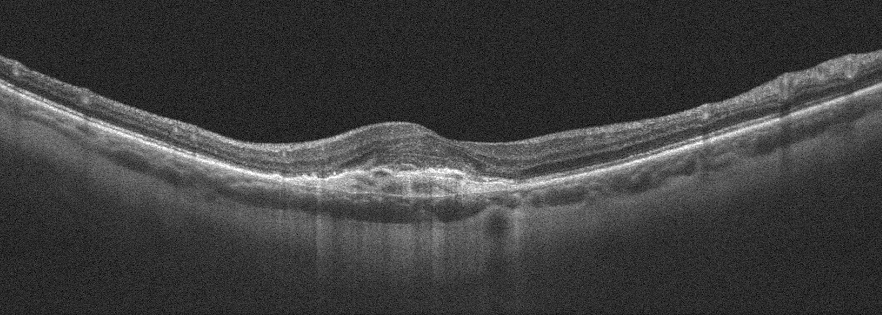
Assessment: AMD.